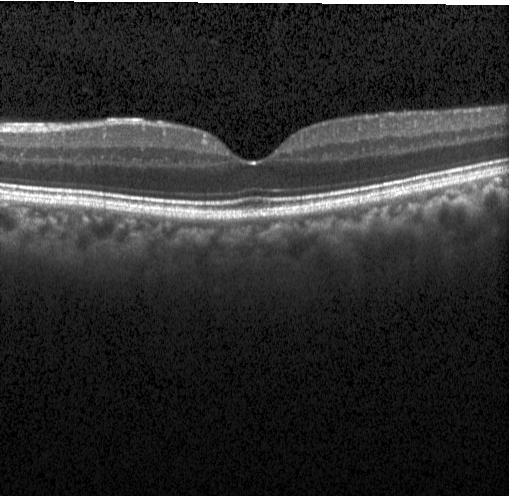
Through the macula; spectral-domain OCT; Heidelberg Spectralis; OCT B-scan. Diagnosis: neither choroidal neovascularization, diabetic macular edema, nor drusen.